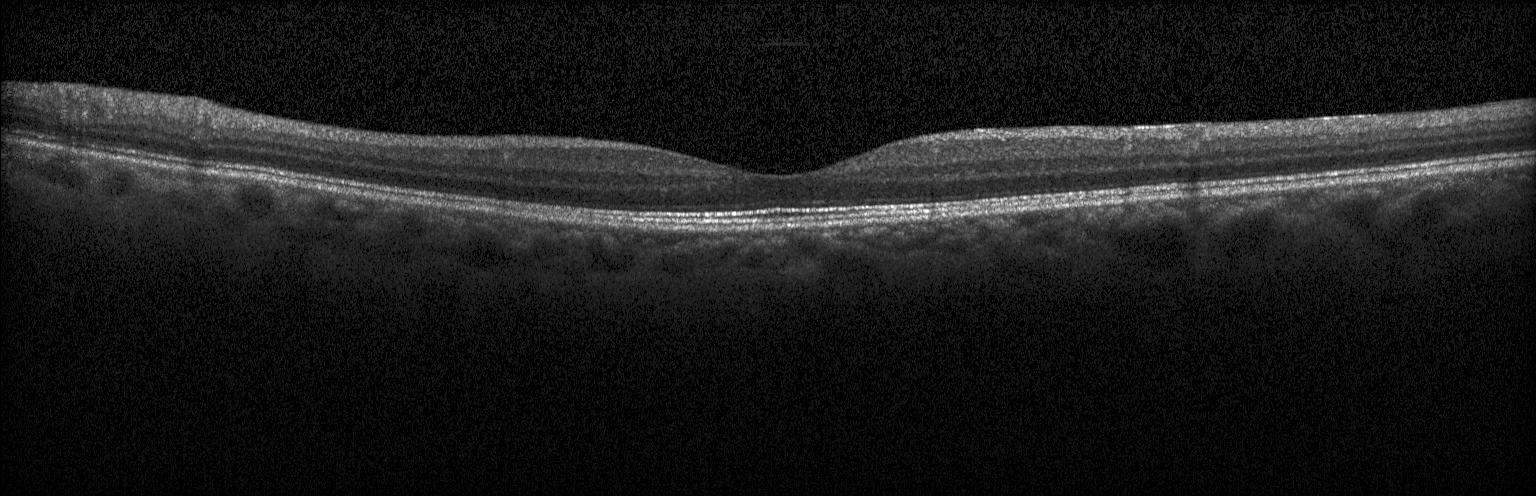 Macular scan; OCT line scan
Impression: no choroidal neovascularization, no diabetic macular edema, and no drusen.